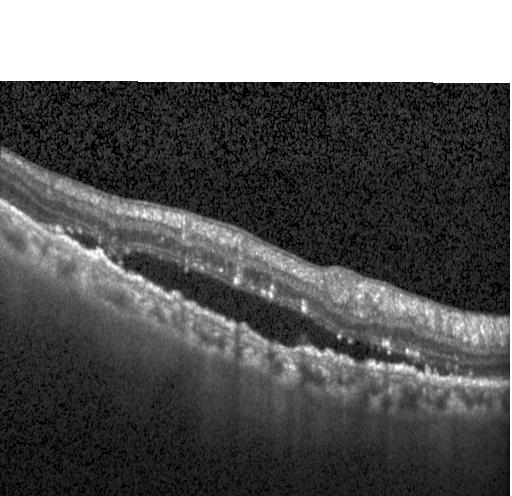

Finding: a choroidal neovascular membrane.